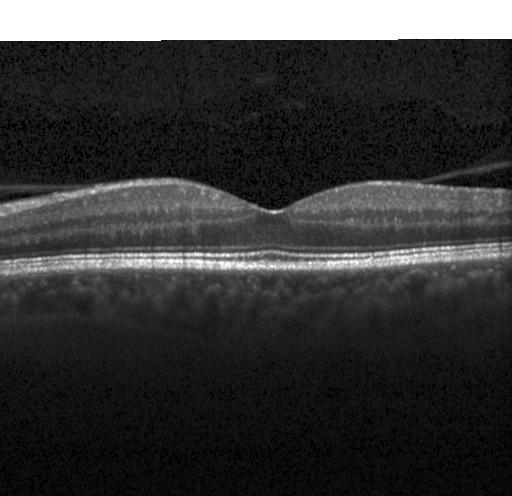 Through the macula · OCT B-scan · Heidelberg Spectralis OCT system · spectral-domain optical coherence tomography. Assessment: no choroidal neovascularization, no diabetic macular edema, and no drusen.